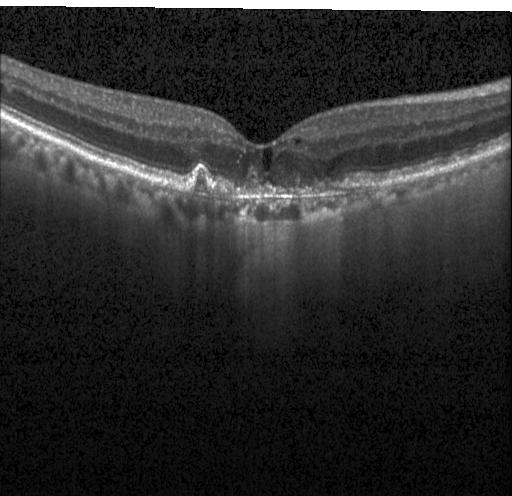 Macular OCT: CNV.